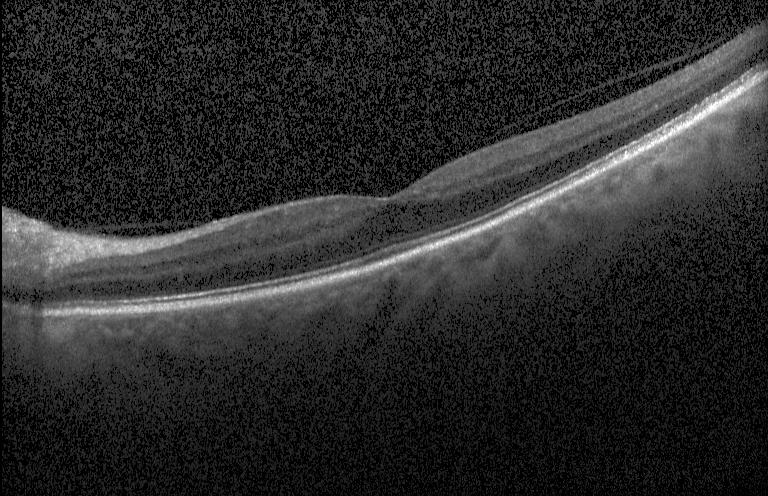

Fovea-centered; spectral-domain optical coherence tomography; optical coherence tomography B-scan. The scan shows no choroidal neovascularization, no diabetic macular edema, and no drusen.